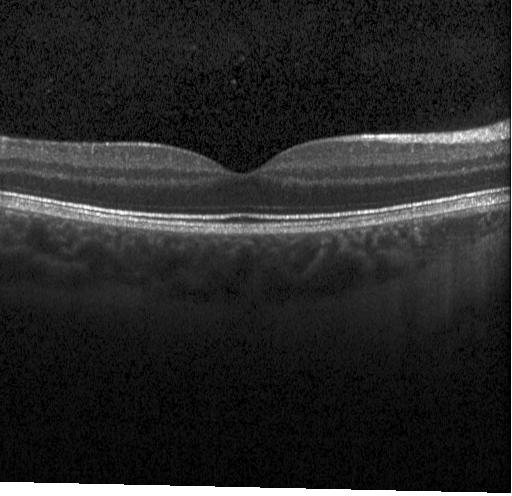

Optical coherence tomography B-scan.
Macular OCT: no choroidal neovascularization, no diabetic macular edema, and no drusen.